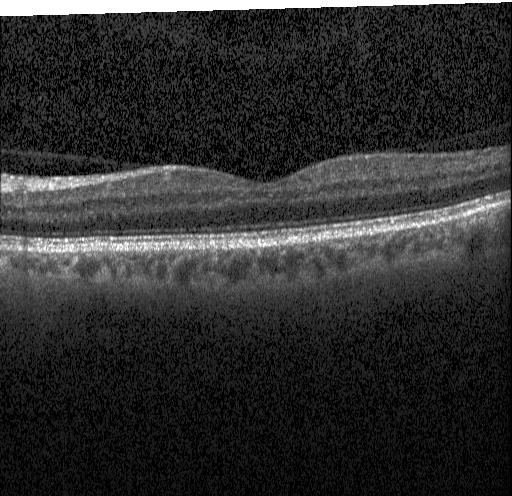

Dx: no choroidal neovascularization, no diabetic macular edema, and no drusen.